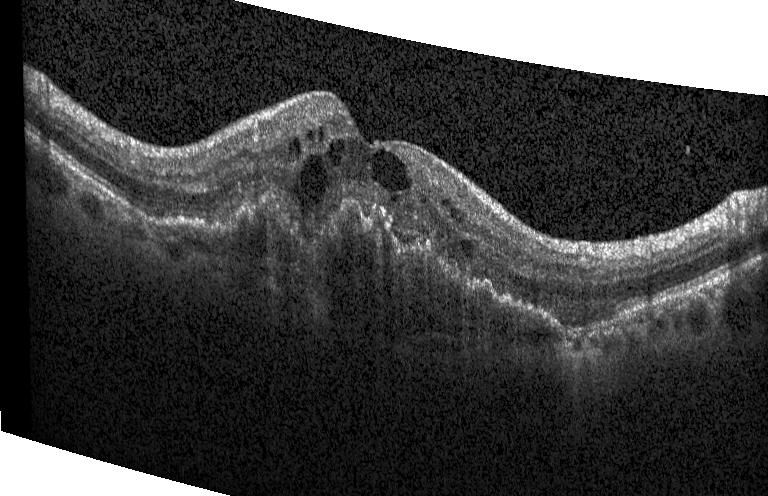
Macular OCT: a choroidal neovascular membrane.